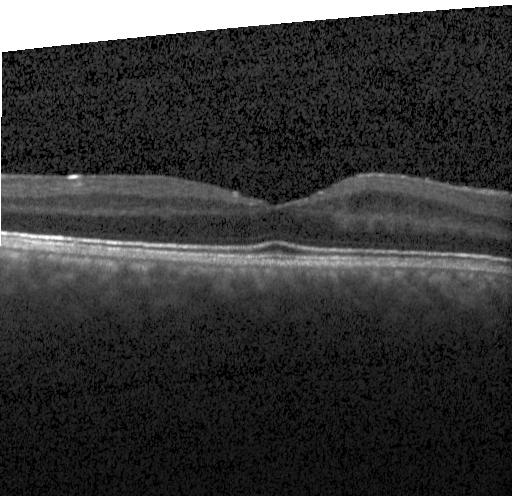
Heidelberg Spectralis OCT system, horizontal scan through the fovea, spectral-domain optical coherence tomography, optical coherence tomography B-scan
Diagnosis: DME.